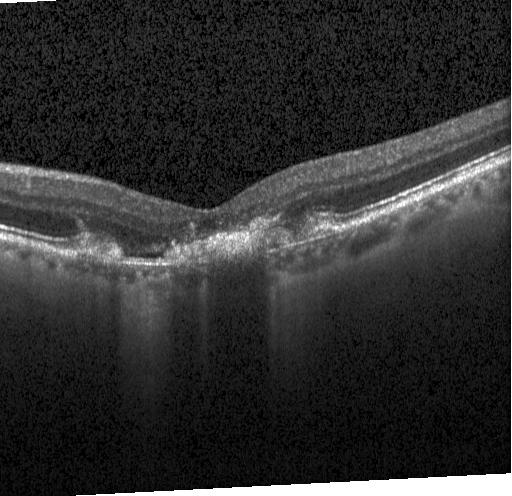 The scan shows choroidal neovascularization (CNV).